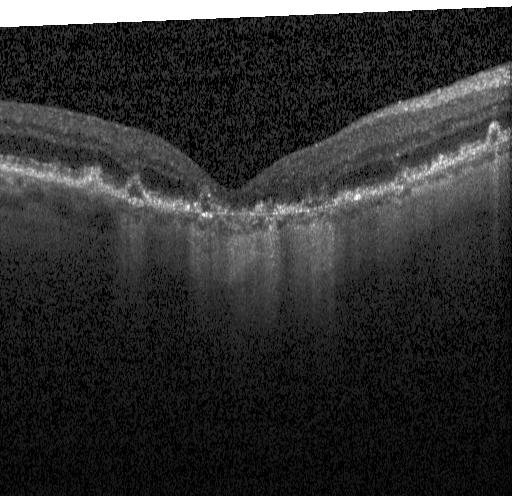

The scan shows choroidal neovascularization (CNV).